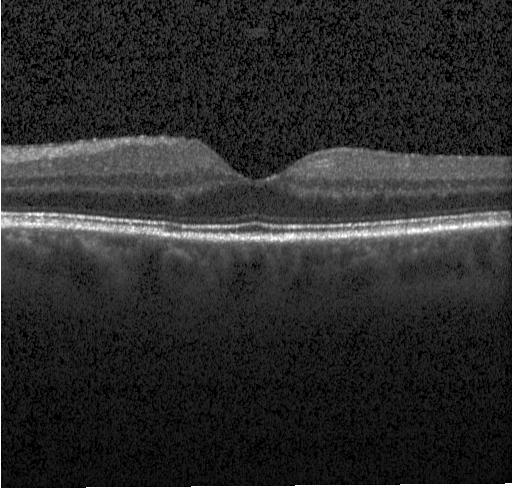

SD-OCT · through the macula · Heidelberg Spectralis · OCT B-scan — Impression: neither choroidal neovascularization, diabetic macular edema, nor drusen.